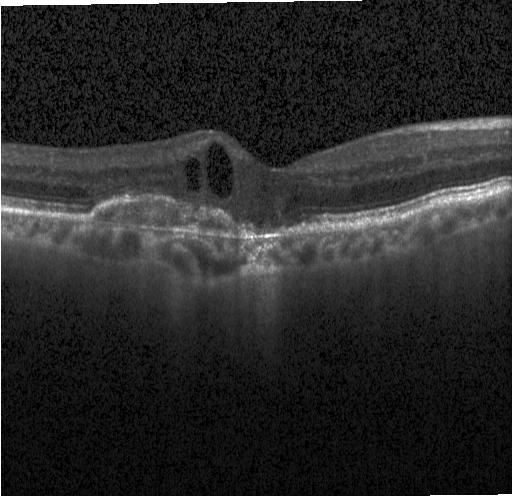 Impression: CNV.